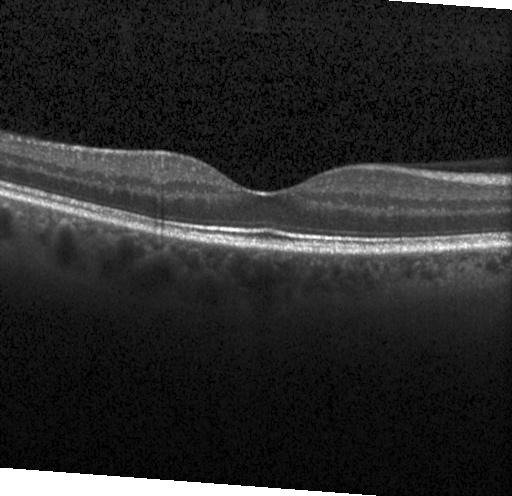
Optical coherence tomography B-scan, spectral-domain optical coherence tomography, acquired on a Heidelberg Spectralis.
Assessment: no choroidal neovascularization, diabetic macular edema, or drusen.